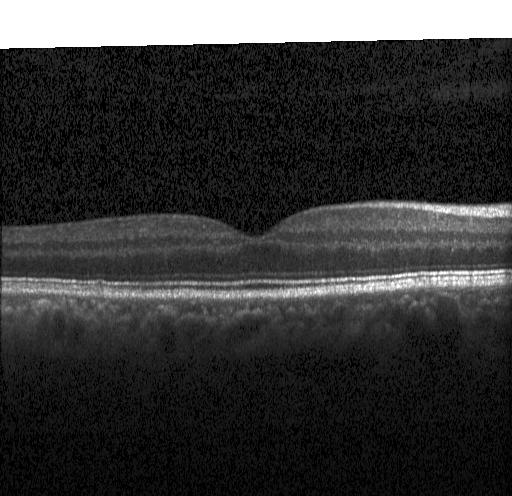 Spectral-domain OCT B-scan: no choroidal neovascularization, diabetic macular edema, or drusen.